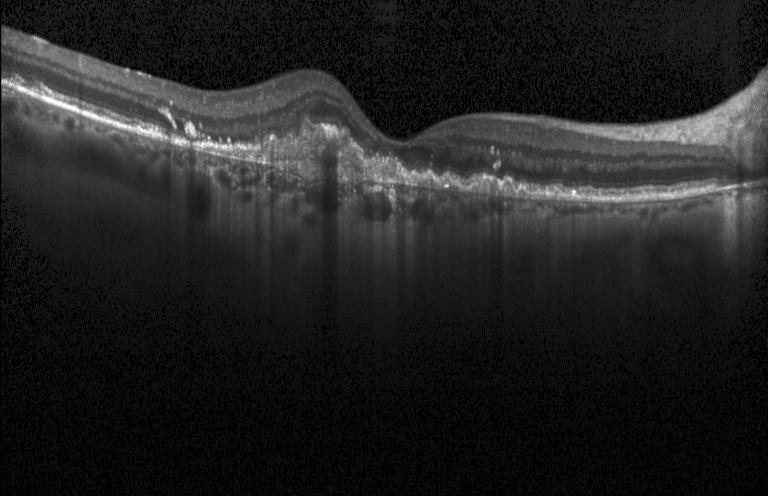

Spectral-domain optical coherence tomography, retinal OCT B-scan, horizontal scan through the fovea. OCT finding: CNV.